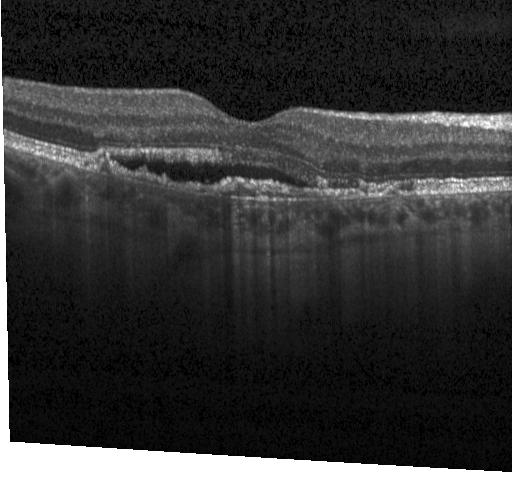

Optical coherence tomography B-scan — Impression: a choroidal neovascular membrane.